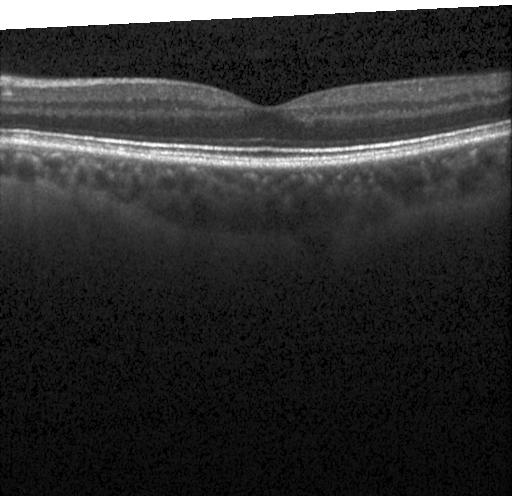
Spectral-domain OCT, OCT B-scan — Impression: no evidence of choroidal neovascularization, diabetic macular edema, or drusen.